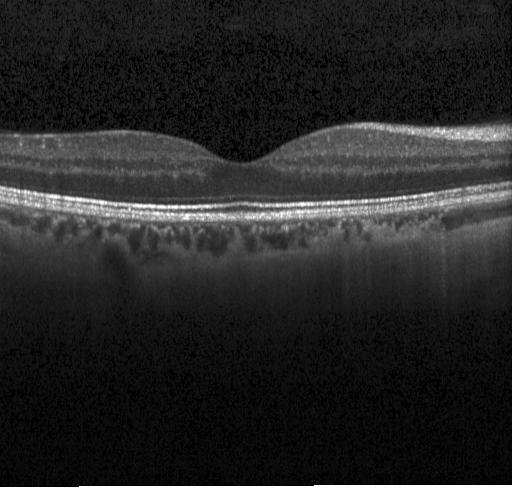 Through the macula · spectral-domain optical coherence tomography · Heidelberg Spectralis OCT system · OCT line scan.
OCT finding: no evidence of CNV, DME, or drusen.